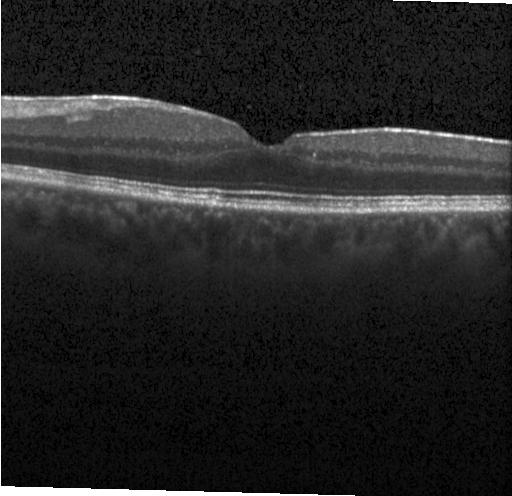 Macular scan. Heidelberg Spectralis OCT system. OCT B-scan. SD-OCT.
Finding: no choroidal neovascularization, no diabetic macular edema, and no drusen.